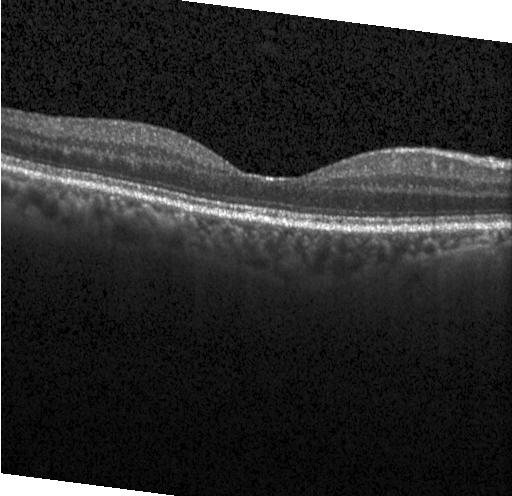

Retinal OCT B-scan — No choroidal neovascularization, diabetic macular edema, or drusen.